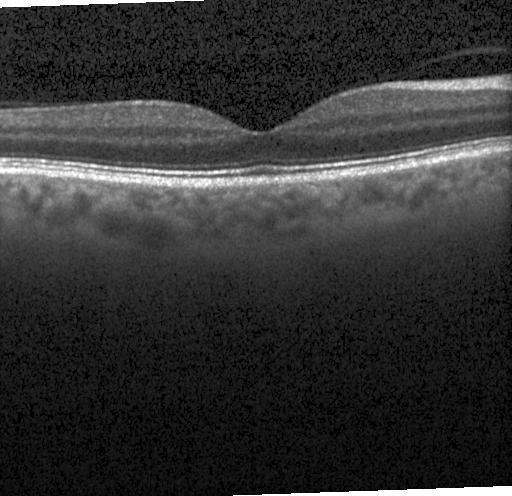 This B-scan demonstrates no choroidal neovascularization, no diabetic macular edema, and no drusen.